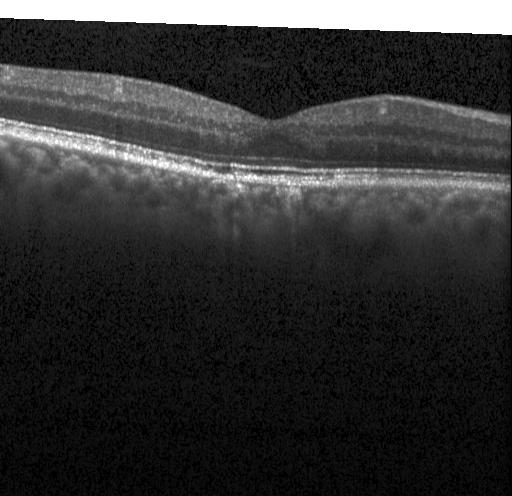

Through the macula; spectral-domain optical coherence tomography; OCT line scan — Dx: no choroidal neovascularization, diabetic macular edema, or drusen.